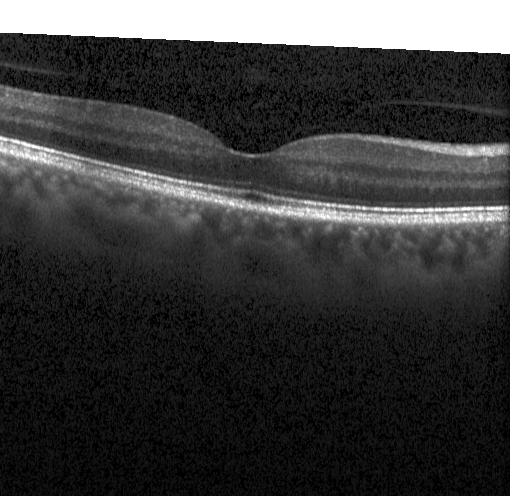
Impression: no choroidal neovascularization, no diabetic macular edema, and no drusen.